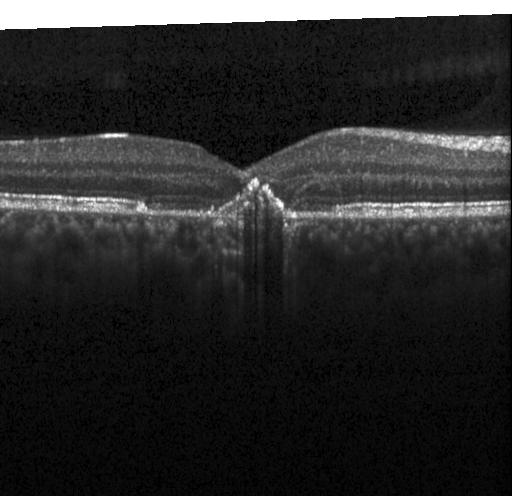

Optical coherence tomography scan. Impression: choroidal neovascularization.